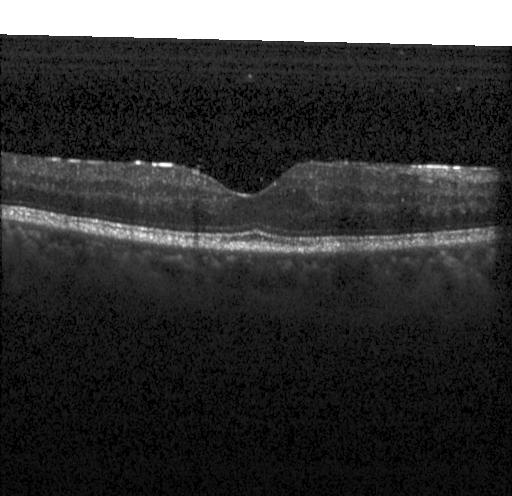
Optical coherence tomography B-scan. Acquired on a Heidelberg Spectralis. Centered on the fovea.
Diagnosis: no CNV, no DME, and no drusen.